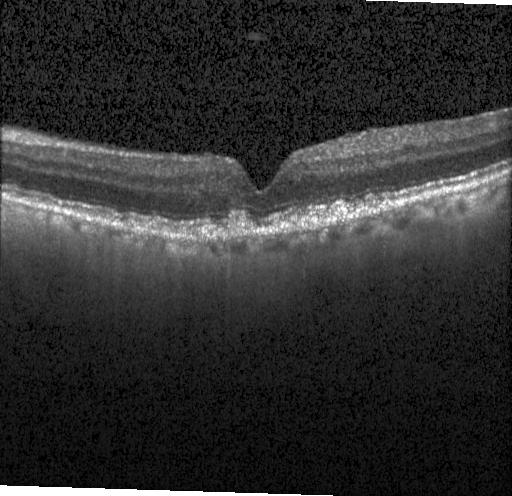 Optical coherence tomography scan; spectral-domain optical coherence tomography.
Dx: multiple drusen.